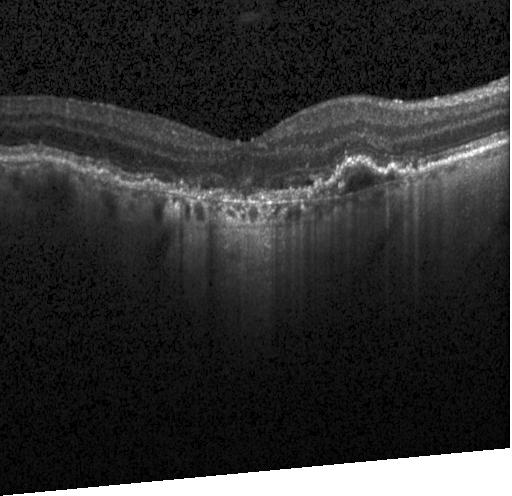 OCT scan showing CNV.